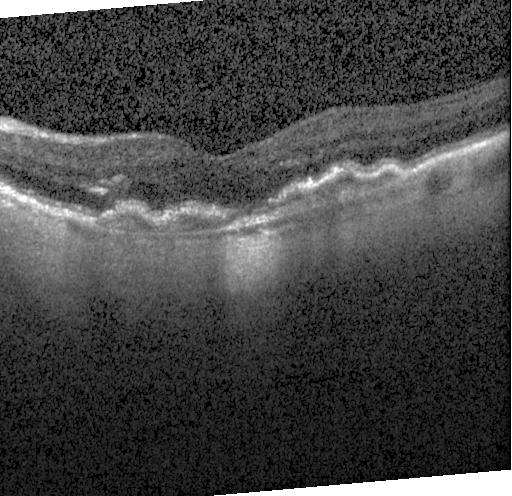

SD-OCT · Heidelberg Spectralis OCT system · OCT B-scan · fovea-centered — Macular OCT: a choroidal neovascular membrane.